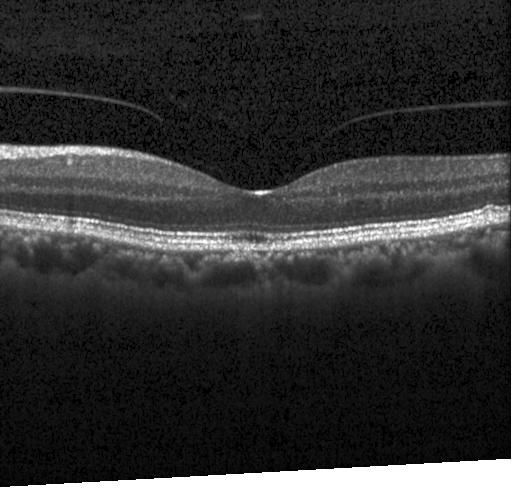

Macular OCT: no choroidal neovascularization, no diabetic macular edema, and no drusen.